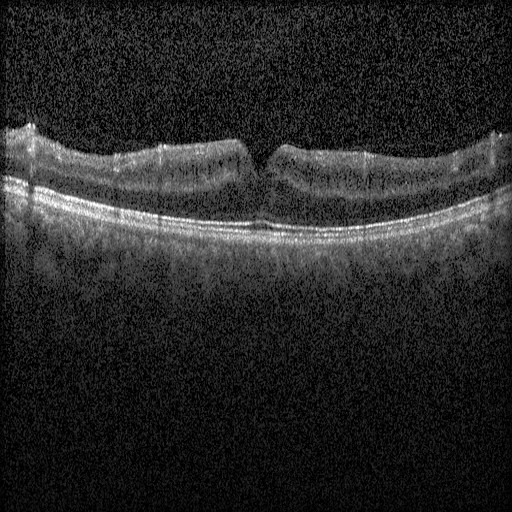
Finding: DME.